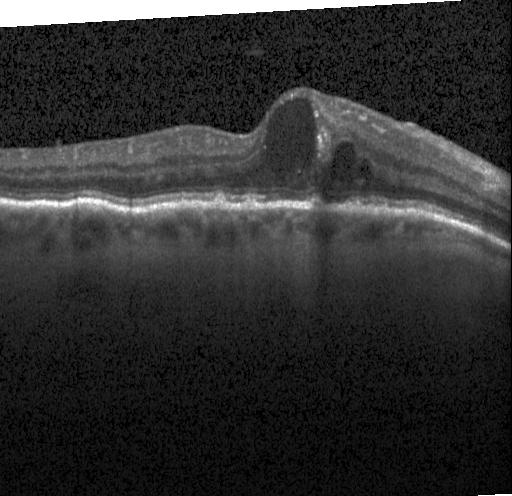 Macular scan; retinal OCT B-scan; spectral-domain optical coherence tomography; instrument: Heidelberg Spectralis — Finding: choroidal neovascularization.